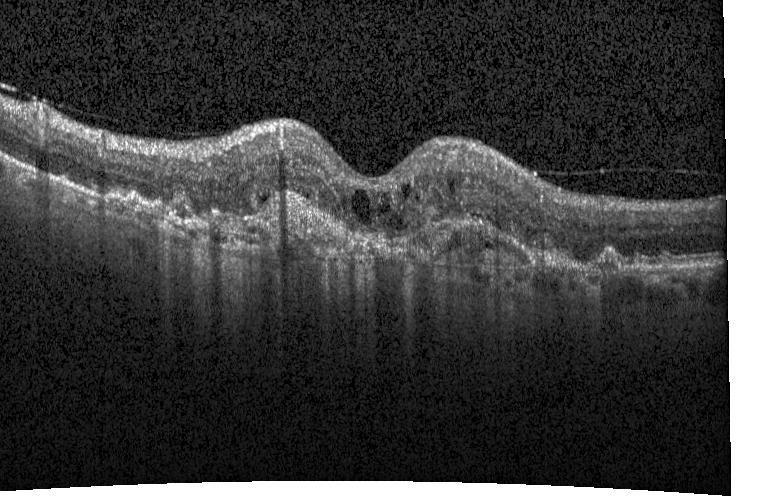 Spectral-domain OCT; instrument: Heidelberg Spectralis; centered on the fovea; retinal OCT B-scan — This B-scan demonstrates a choroidal neovascular membrane.